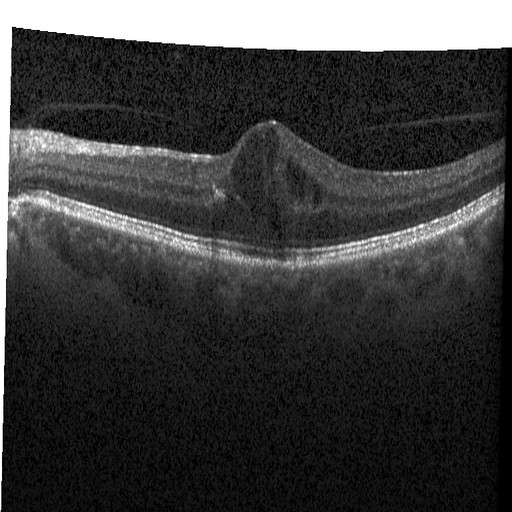
Retinal OCT cross-section. Spectral-domain OCT. Impression: diabetic macular edema.